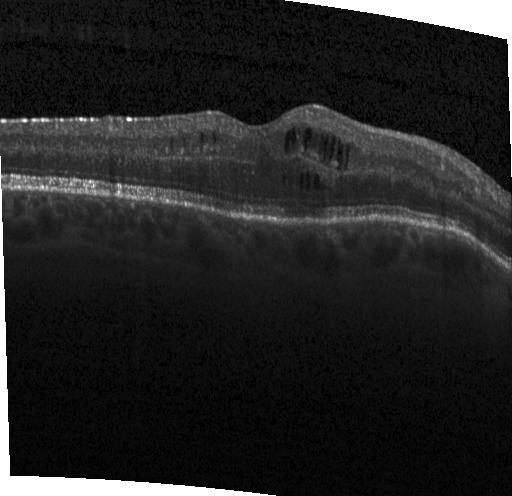

SD-OCT; OCT B-scan.
Finding: diabetic macular edema (DME).